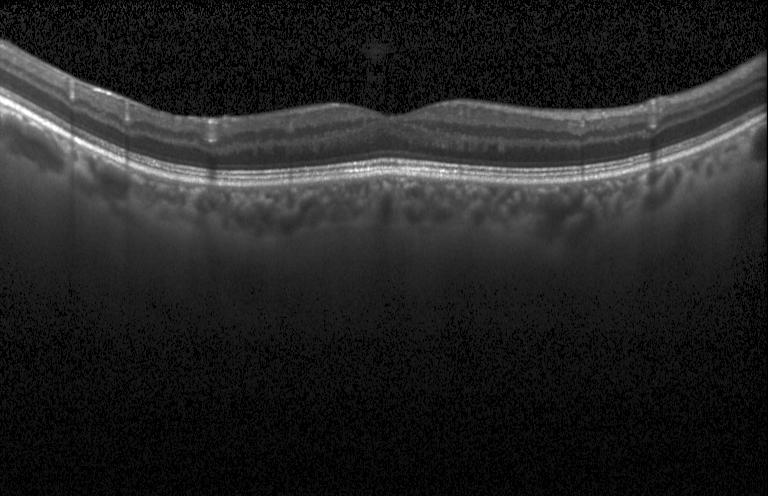
Heidelberg Spectralis OCT system; OCT B-scan; horizontal scan through the fovea
Impression: no CNV, DME, or drusen.